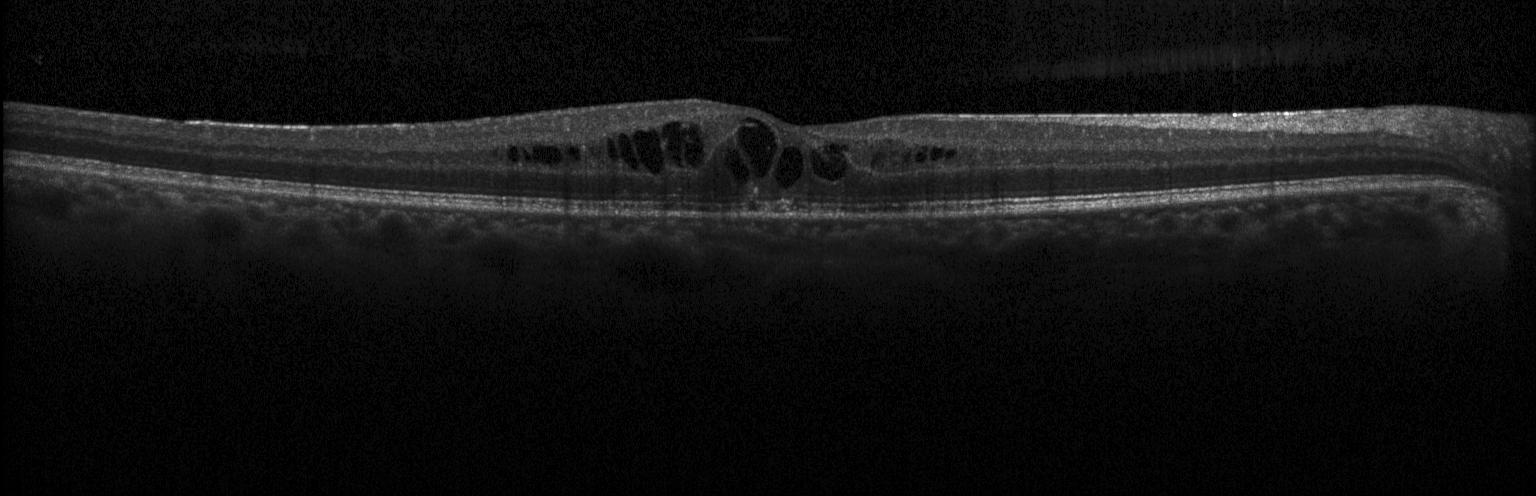 Through the macula · retinal OCT cross-section — Macular OCT: diabetic macular edema (DME).